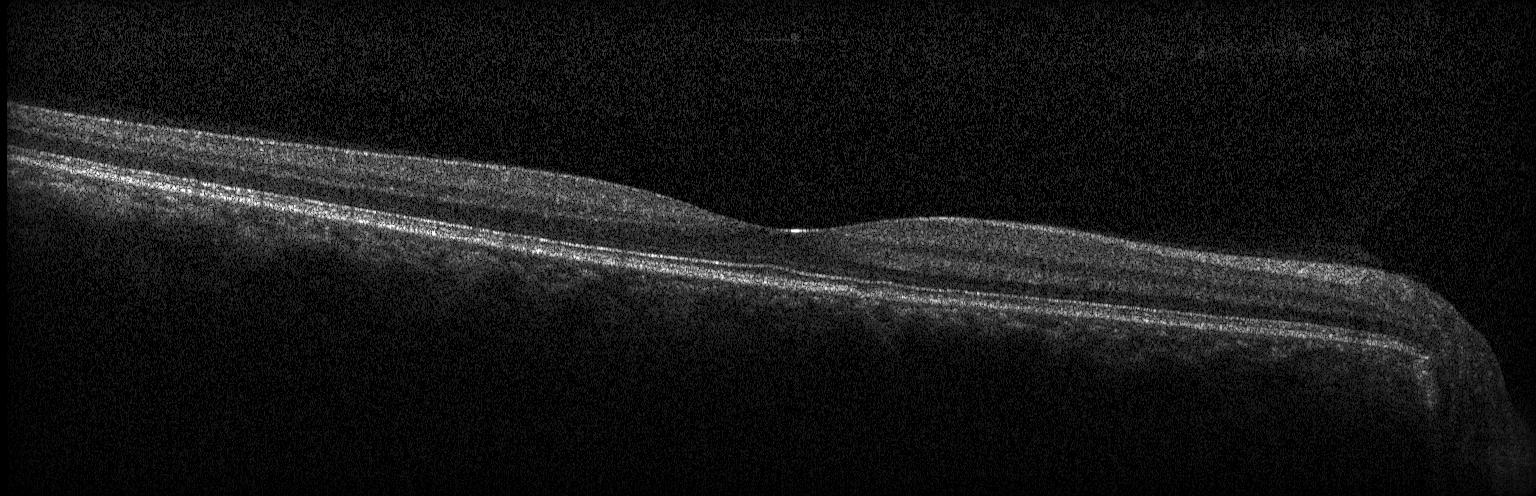
Fovea-centered; OCT B-scan — Assessment: neither choroidal neovascularization, diabetic macular edema, nor drusen.